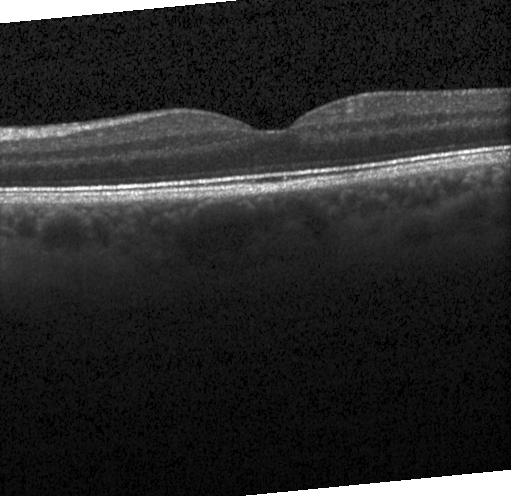

Retinal OCT cross-section — Impression: neither CNV, DME, nor drusen.